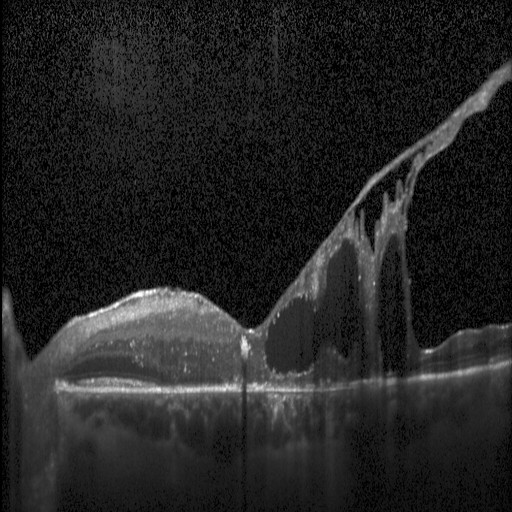
Instrument: Heidelberg Spectralis · SD-OCT · through the macula · optical coherence tomography scan. The scan shows diabetic macular edema (DME).